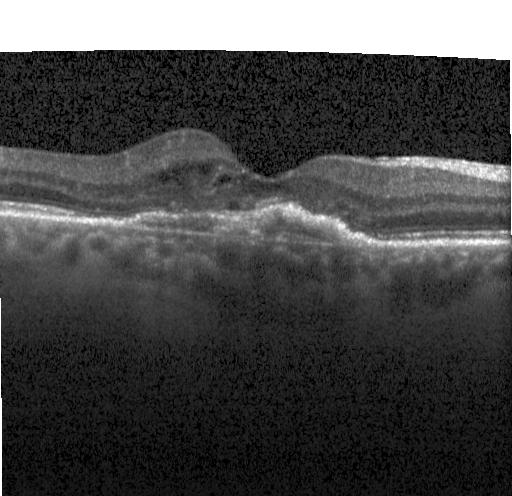
Assessment: a choroidal neovascular membrane.